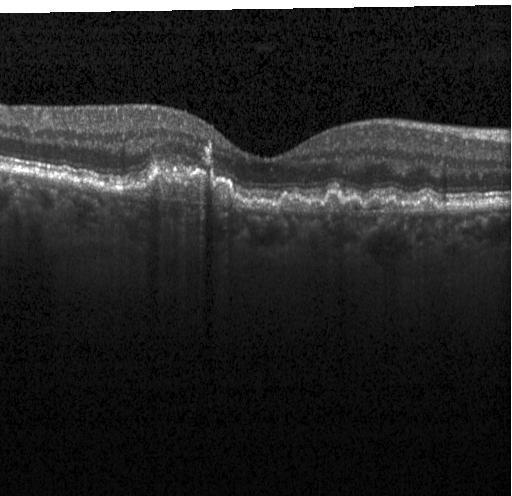

Impression: choroidal neovascularization.